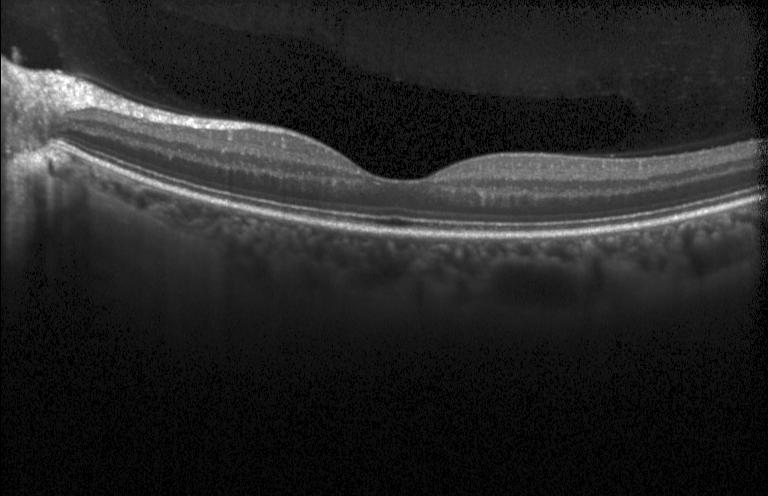 OCT line scan. No choroidal neovascularization, diabetic macular edema, or drusen.